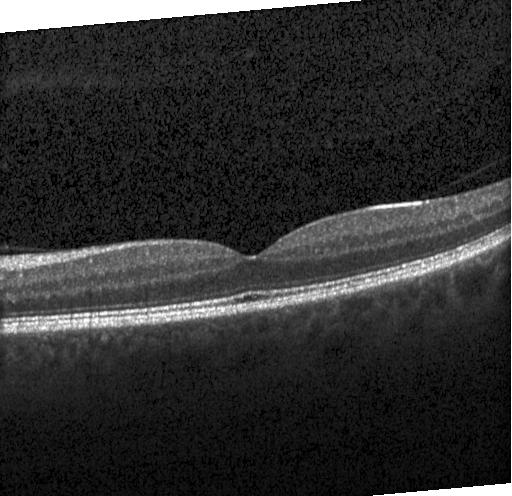
Macular OCT demonstrating no evidence of choroidal neovascularization, diabetic macular edema, or drusen.